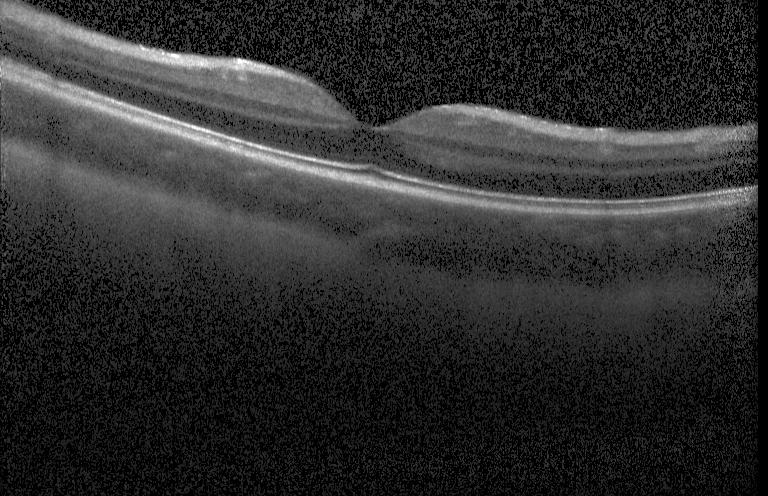 Spectral-domain OCT B-scan: no evidence of choroidal neovascularization, diabetic macular edema, or drusen.